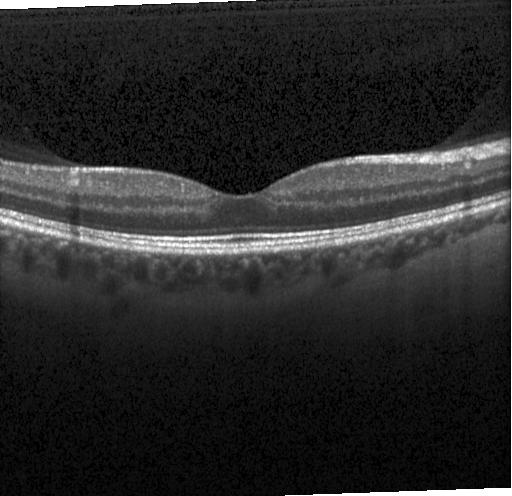
Retinal OCT B-scan — Dx: no CNV, DME, or drusen.